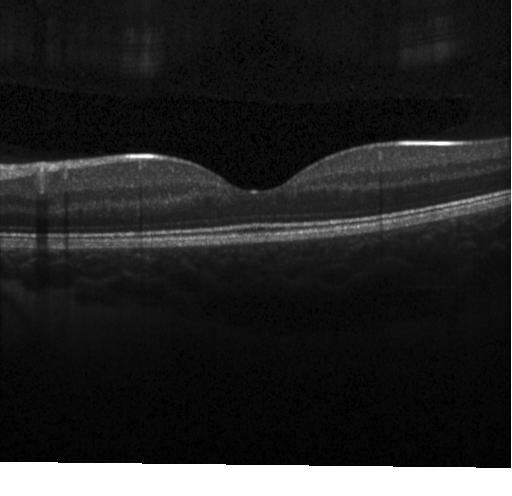 Centered on the fovea, retinal OCT B-scan, acquired on a Heidelberg Spectralis
Finding: no choroidal neovascularization, no diabetic macular edema, and no drusen.